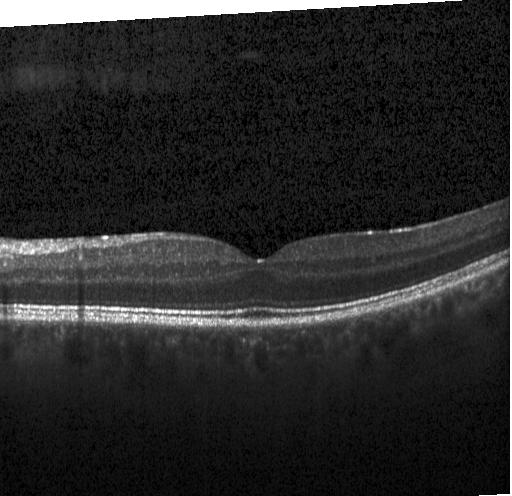
OCT B-scan; instrument: Heidelberg Spectralis; centered on the fovea — The scan shows no evidence of choroidal neovascularization, diabetic macular edema, or drusen.